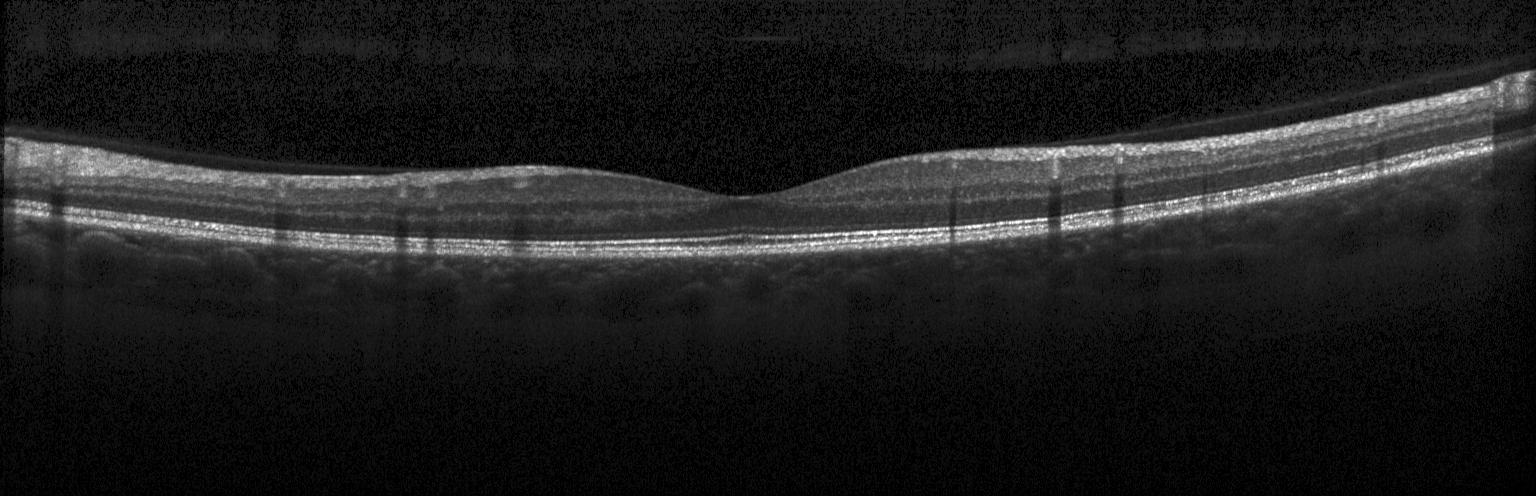

Retinal OCT cross-section — Diagnosis: neither choroidal neovascularization, diabetic macular edema, nor drusen.